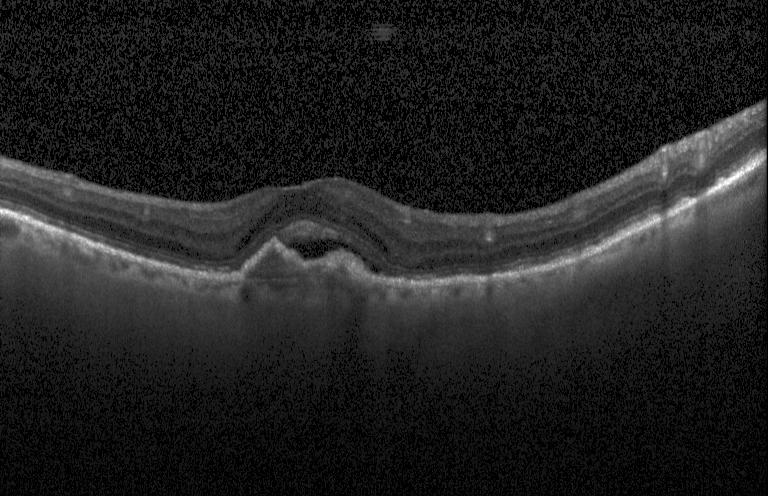 Spectral-domain OCT, horizontal scan through the fovea, retinal OCT cross-section, instrument: Heidelberg Spectralis.
Diagnosis: choroidal neovascularization (CNV).